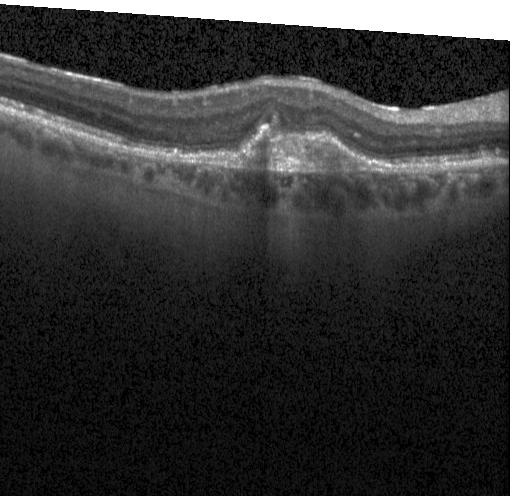
OCT line scan; horizontal scan through the fovea; spectral-domain optical coherence tomography.
A choroidal neovascular membrane.